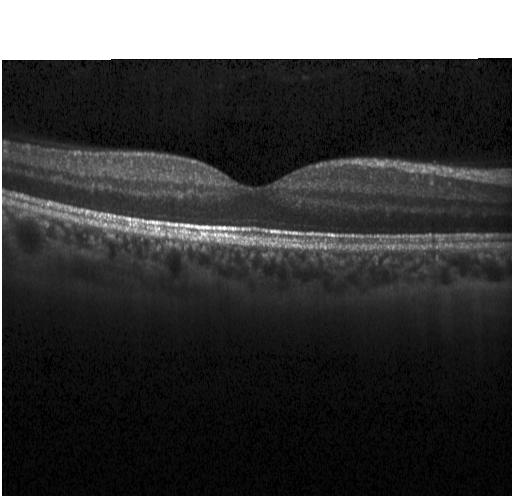
Macular scan · OCT B-scan · instrument: Heidelberg Spectralis · spectral-domain optical coherence tomography
Finding: no CNV, DME, or drusen.